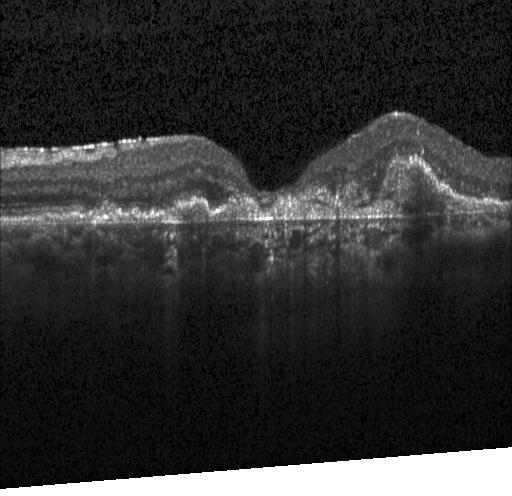

Diagnosis: a choroidal neovascular membrane.